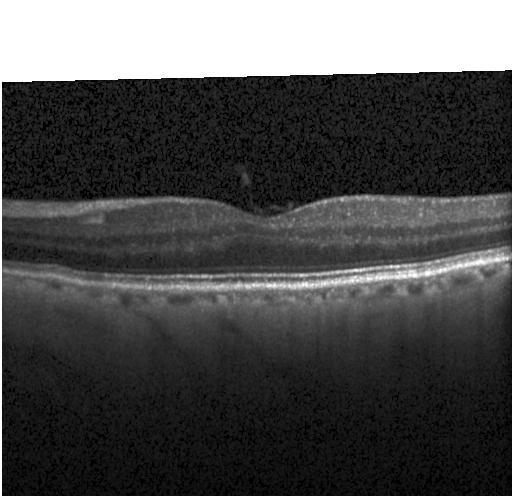 Acquired on a Heidelberg Spectralis; spectral-domain OCT; optical coherence tomography scan. OCT finding: neither choroidal neovascularization, diabetic macular edema, nor drusen.